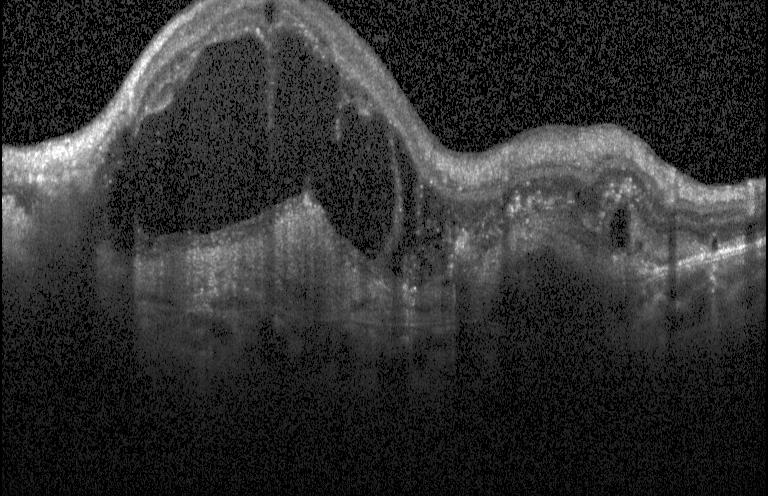
OCT scan showing a choroidal neovascular membrane.